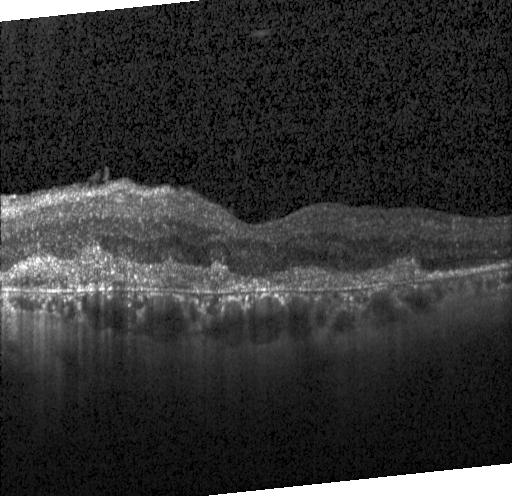 Diagnosis: a choroidal neovascular membrane.